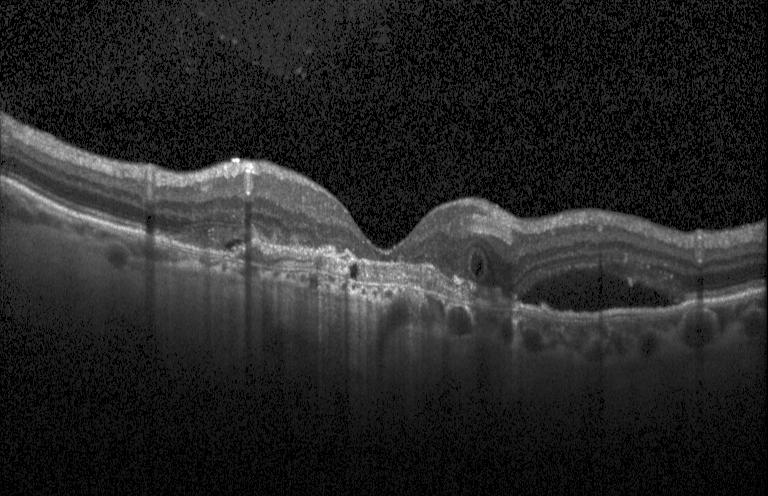
Heidelberg Spectralis OCT system · retinal OCT cross-section · fovea-centered
Dx: a choroidal neovascular membrane.